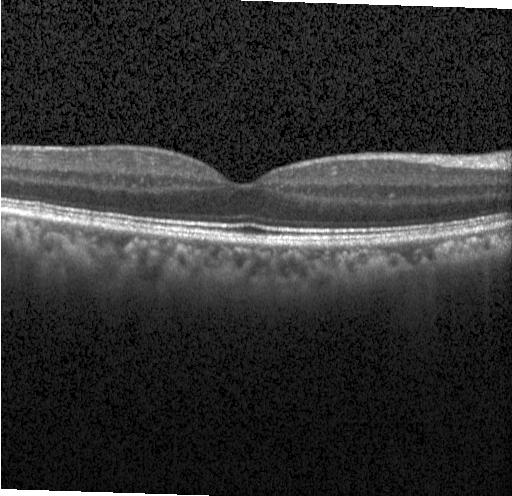

SD-OCT, retinal OCT B-scan, Heidelberg Spectralis OCT system, macular scan
This B-scan demonstrates no choroidal neovascularization, no diabetic macular edema, and no drusen.